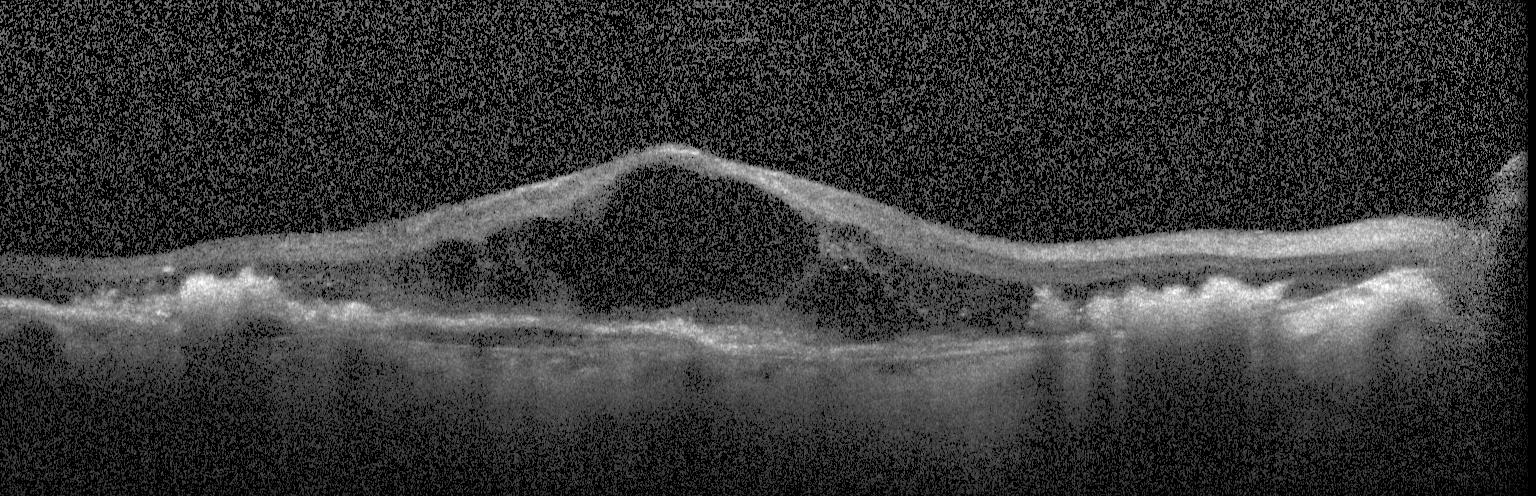
OCT B-scan. Spectral-domain optical coherence tomography. Macular scan. OCT finding: a choroidal neovascular membrane.